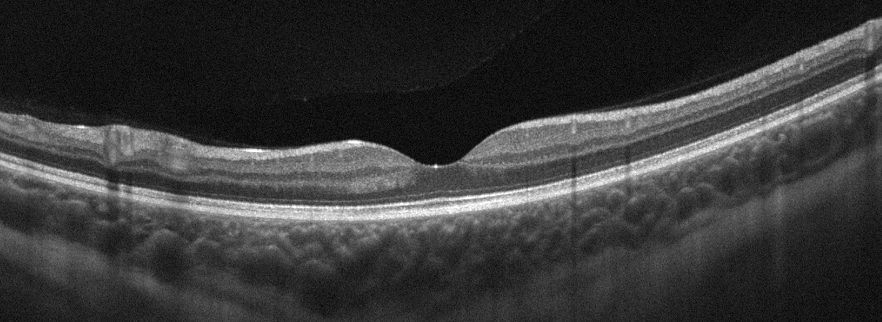 OCT B-scan. OD
OCT finding: absence of AMD, DME, ERM, RAO, RVO, and vitreomacular interface disease.